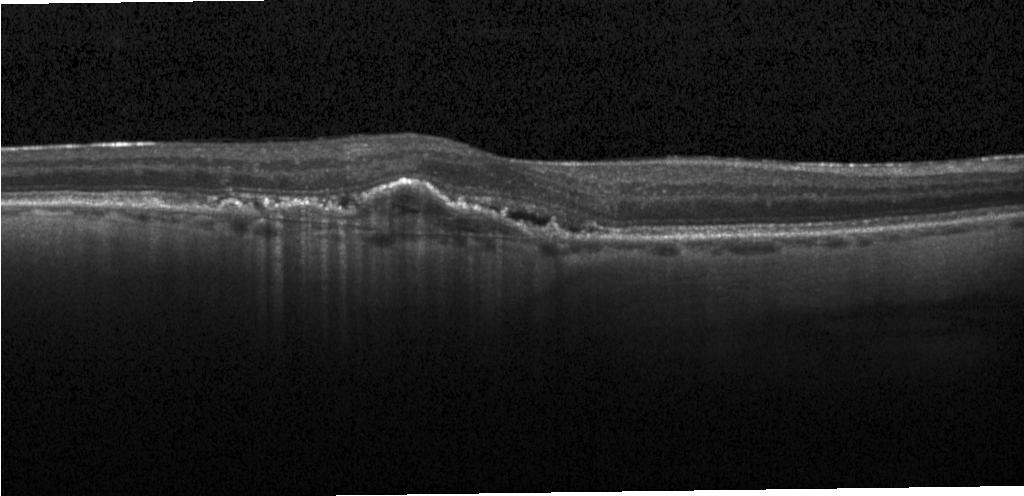 Finding: a choroidal neovascular membrane.